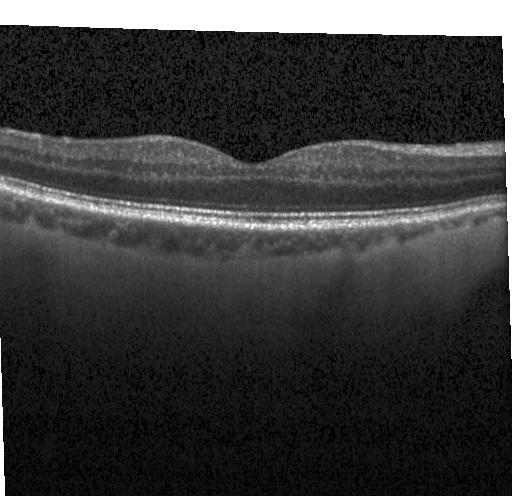 Optical coherence tomography B-scan. Impression: no choroidal neovascularization, no diabetic macular edema, and no drusen.